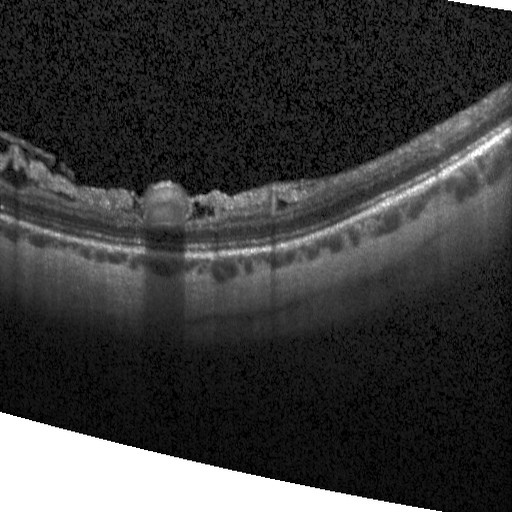

Optical coherence tomography scan. Heidelberg Spectralis. Spectral-domain optical coherence tomography. Assessment: diabetic macular edema (DME).